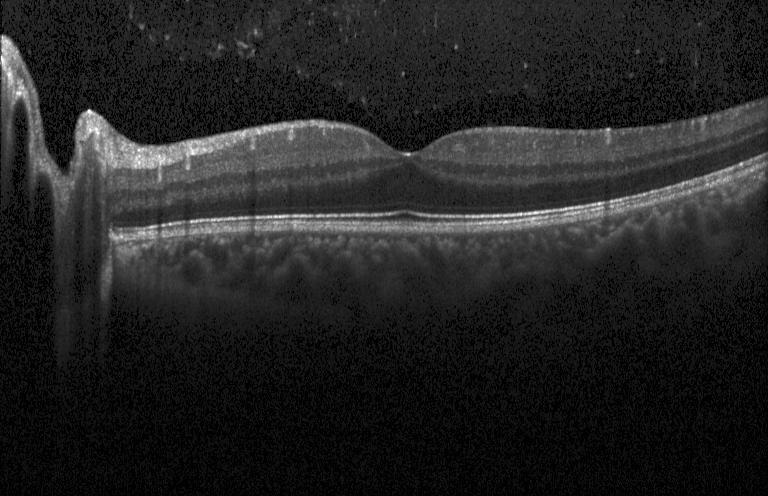

OCT B-scan — Finding: no choroidal neovascularization, no diabetic macular edema, and no drusen.